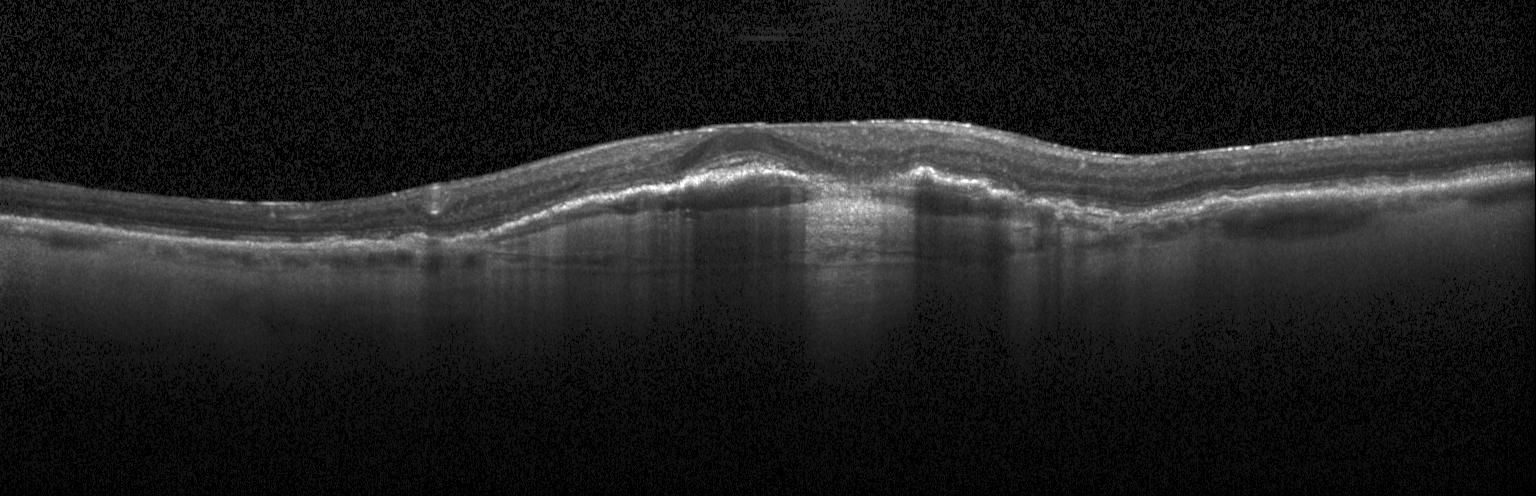
Retinal OCT B-scan — Macular OCT: a choroidal neovascular membrane.